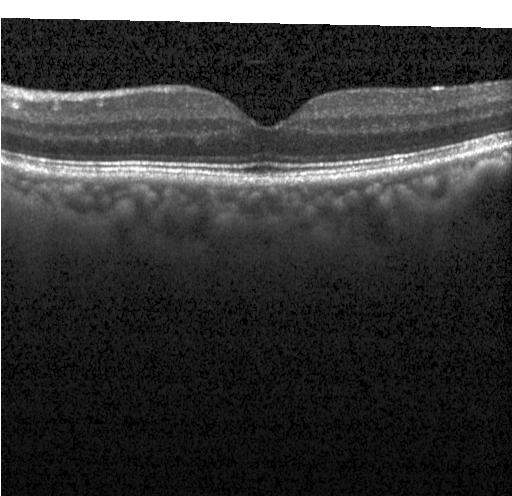

Macular OCT: no choroidal neovascularization, no diabetic macular edema, and no drusen.